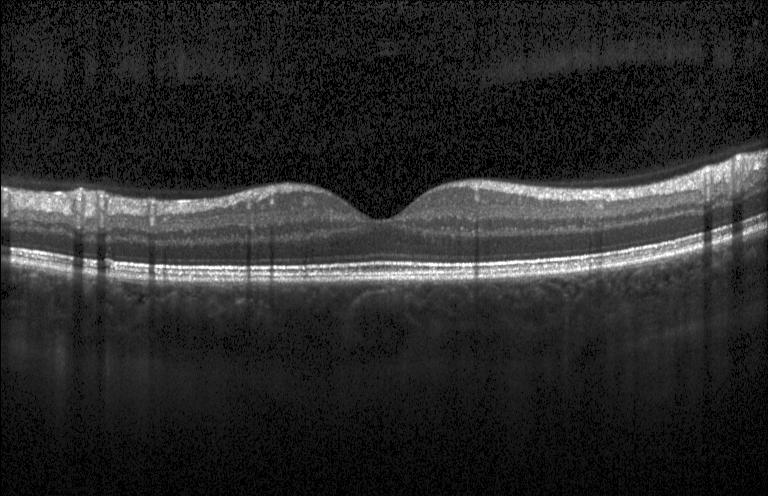
Spectral-domain optical coherence tomography. Fovea-centered. OCT line scan — Diagnosis: no evidence of CNV, DME, or drusen.